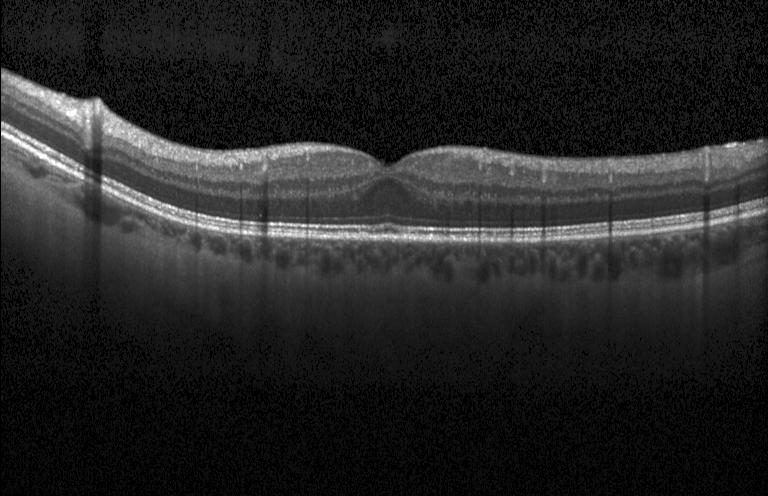 Optical coherence tomography scan · spectral-domain optical coherence tomography · centered on the fovea.
Finding: no evidence of choroidal neovascularization, diabetic macular edema, or drusen.